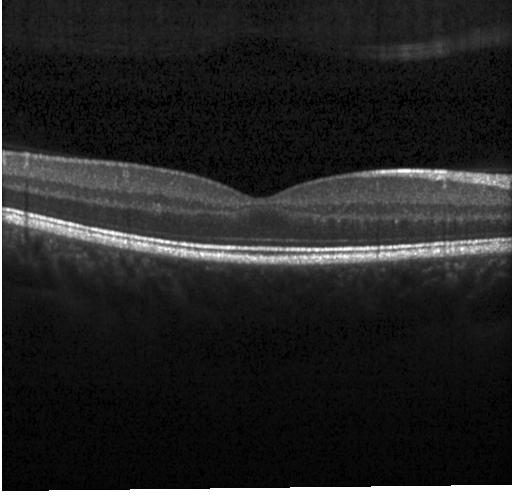

Heidelberg Spectralis, retinal OCT cross-section, spectral-domain OCT — Diagnosis: no choroidal neovascularization, diabetic macular edema, or drusen.